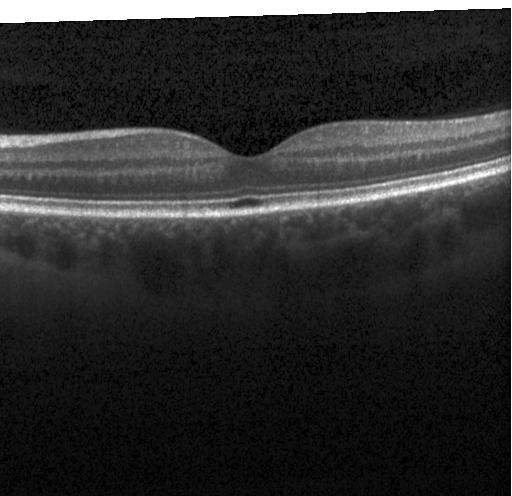
Spectral-domain OCT; optical coherence tomography scan; centered on the fovea
Assessment: no choroidal neovascularization, no diabetic macular edema, and no drusen.